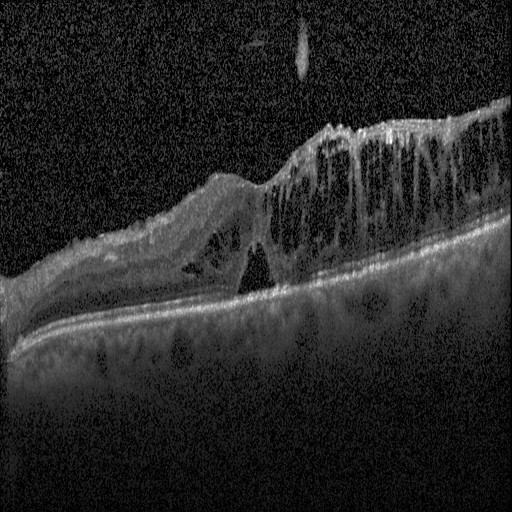
Optical coherence tomography scan, horizontal scan through the fovea. Finding: DME.